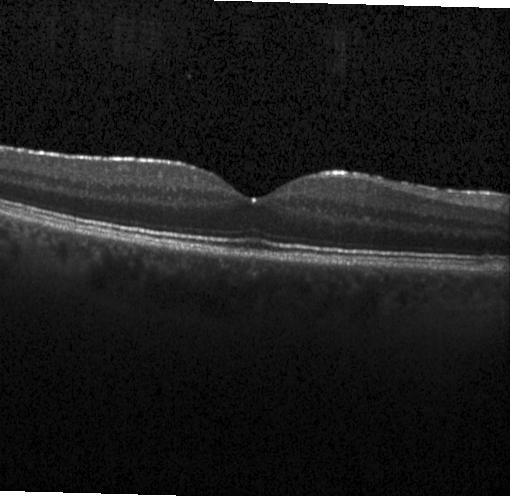

OCT B-scan
Finding: neither choroidal neovascularization, diabetic macular edema, nor drusen.